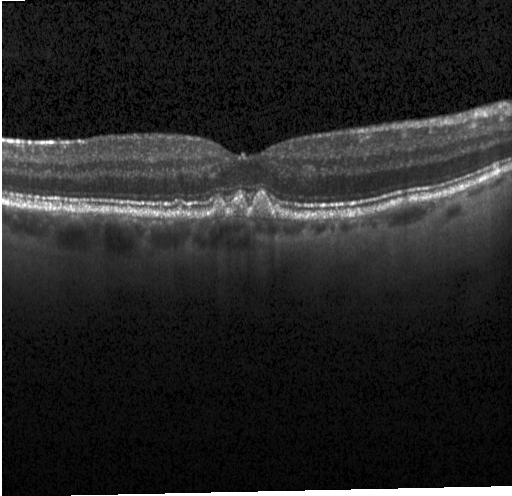

Optical coherence tomography scan
Macular OCT: sub-RPE drusenoid deposits.